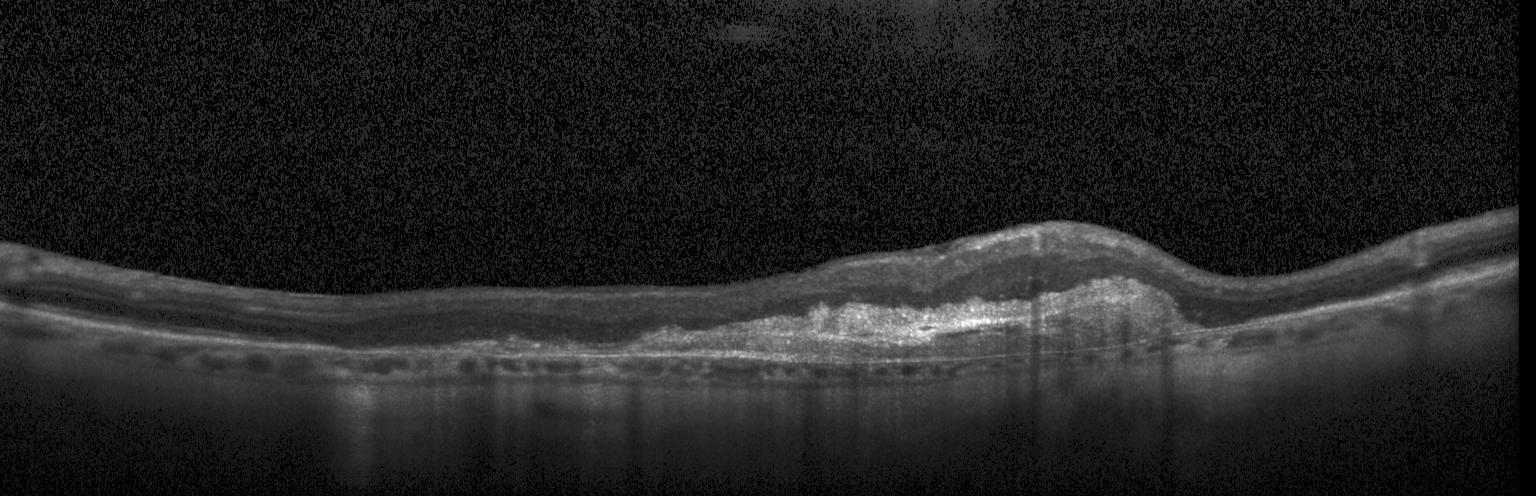

Impression: choroidal neovascularization (CNV).